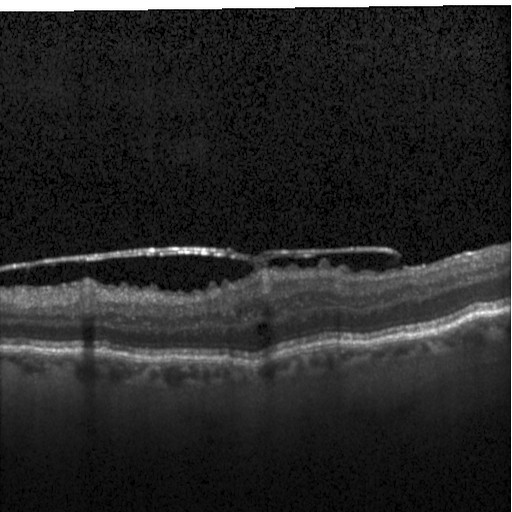
Finding: diabetic macular edema.